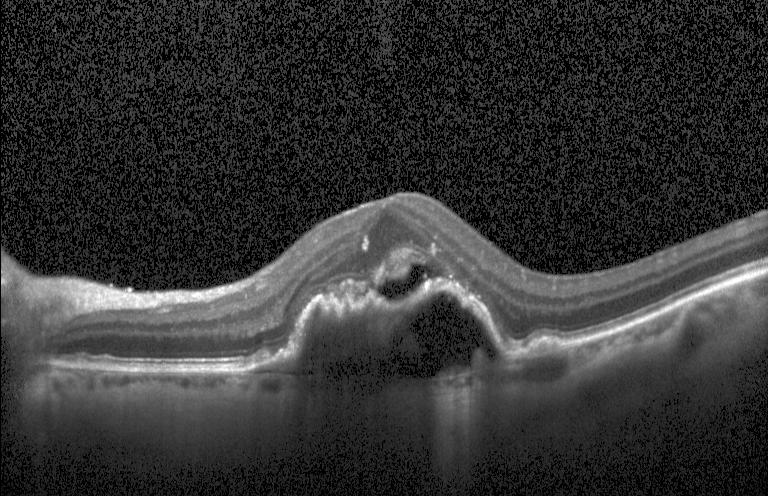 Macular scan. Retinal OCT B-scan — Finding: a choroidal neovascular membrane.